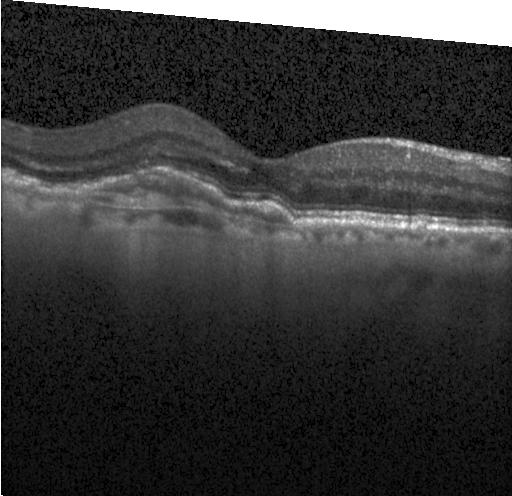
SD-OCT. Heidelberg Spectralis. Optical coherence tomography B-scan. Dx: a choroidal neovascular membrane.